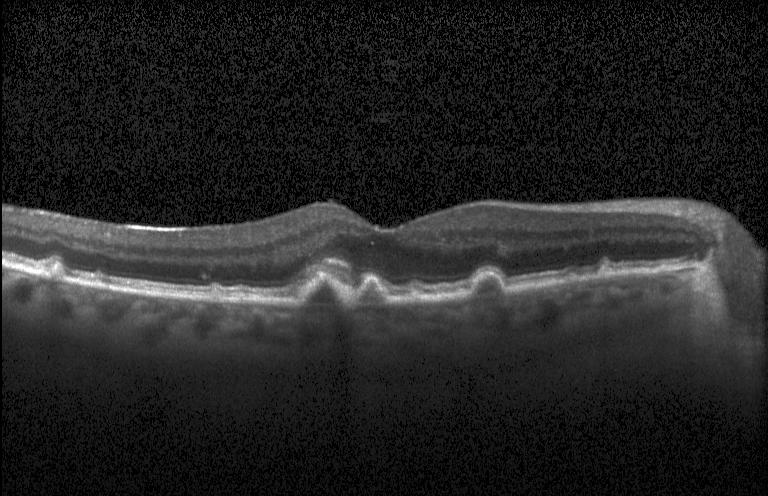 OCT line scan — Finding: multiple drusen.